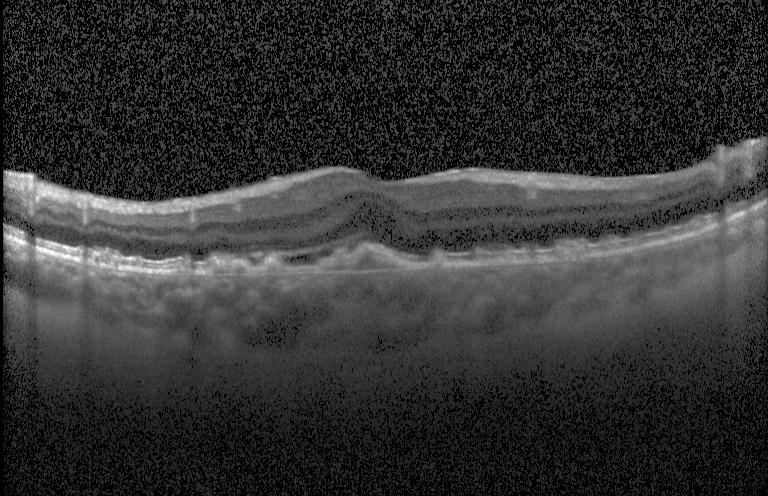

Optical coherence tomography scan; acquired on a Heidelberg Spectralis — Dx: choroidal neovascularization.